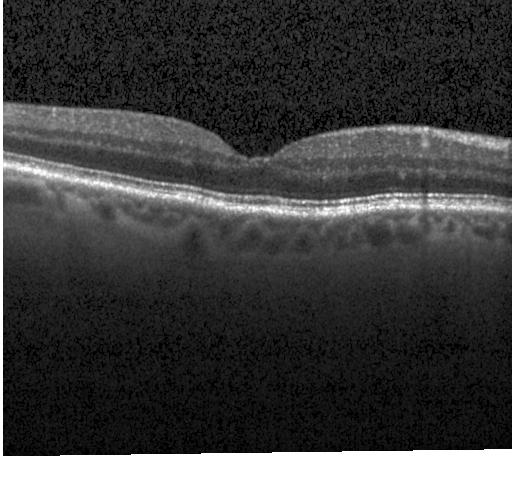
Centered on the fovea · Heidelberg Spectralis OCT system · optical coherence tomography B-scan · spectral-domain OCT.
Impression: neither choroidal neovascularization, diabetic macular edema, nor drusen.